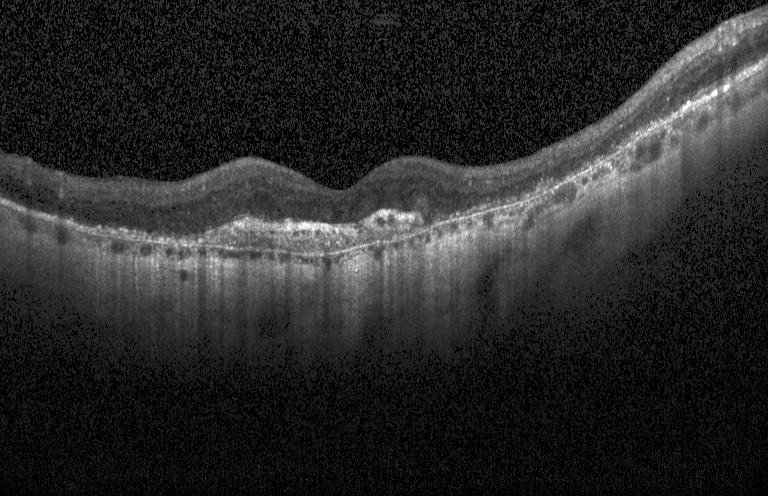 Diagnosis: CNV.